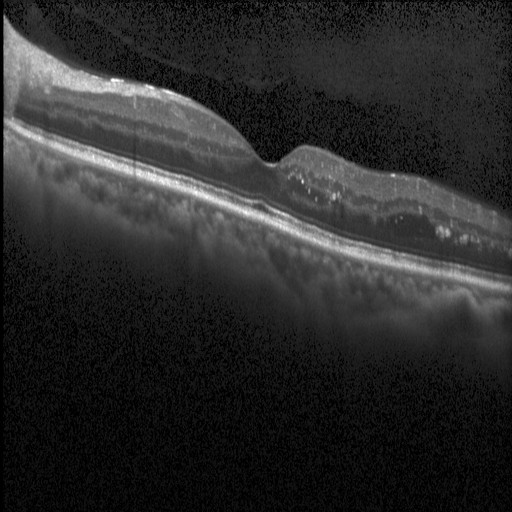

OCT B-scan showing diabetic macular edema (DME).